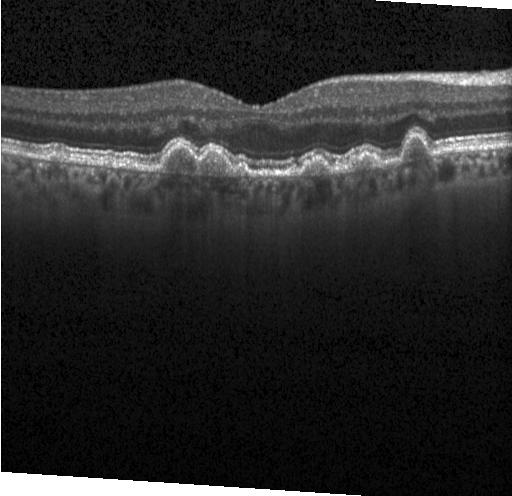

Optical coherence tomography B-scan. Acquired on a Heidelberg Spectralis. Spectral-domain optical coherence tomography. Horizontal scan through the fovea.
Impression: sub-RPE drusenoid deposits.